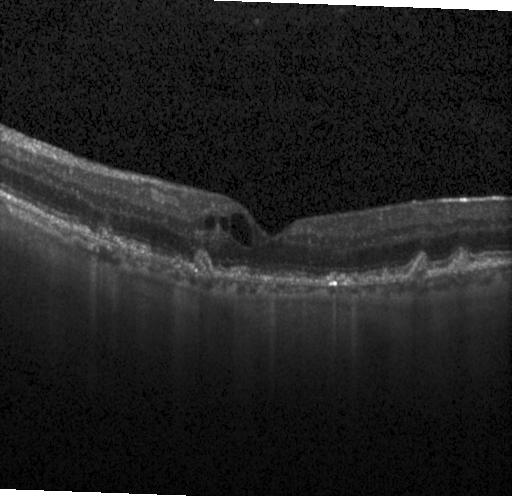
Horizontal scan through the fovea · Heidelberg Spectralis OCT system · SD-OCT · retinal OCT cross-section — A choroidal neovascular membrane.